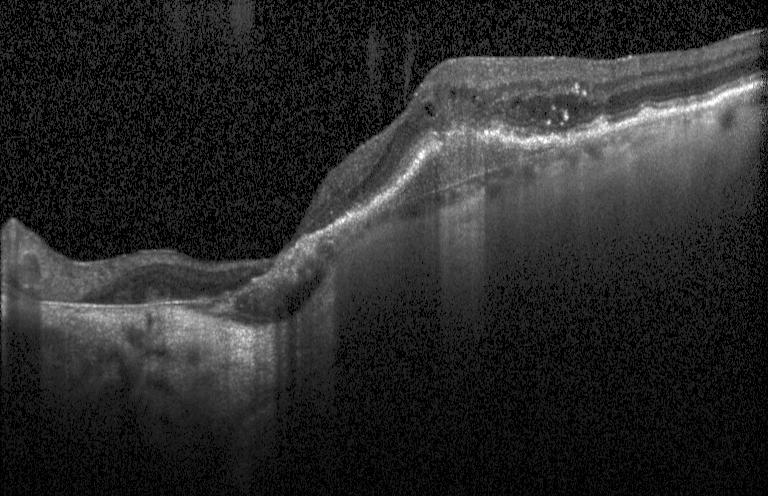 Diagnosis: choroidal neovascularization (CNV).